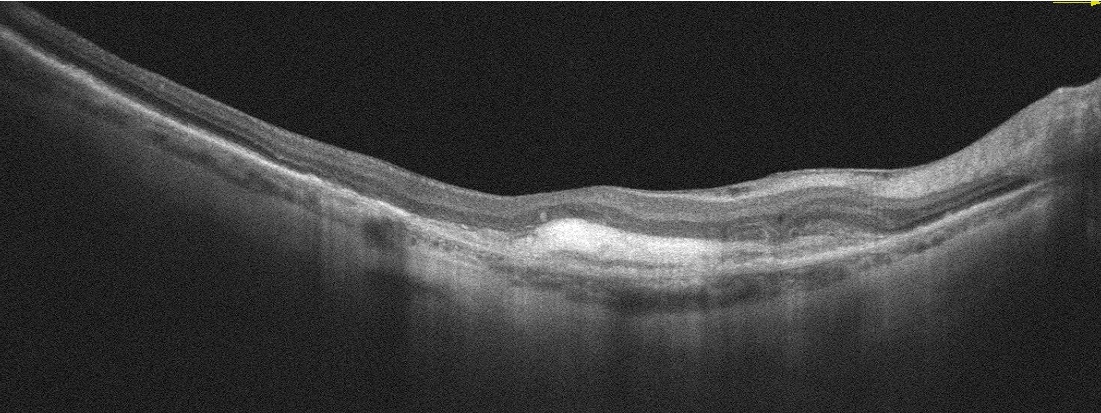
Instrument: Optovue Avanti RTVue XR. Fovea-centered. Optical coherence tomography scan — Dx: age-related macular degeneration (AMD).